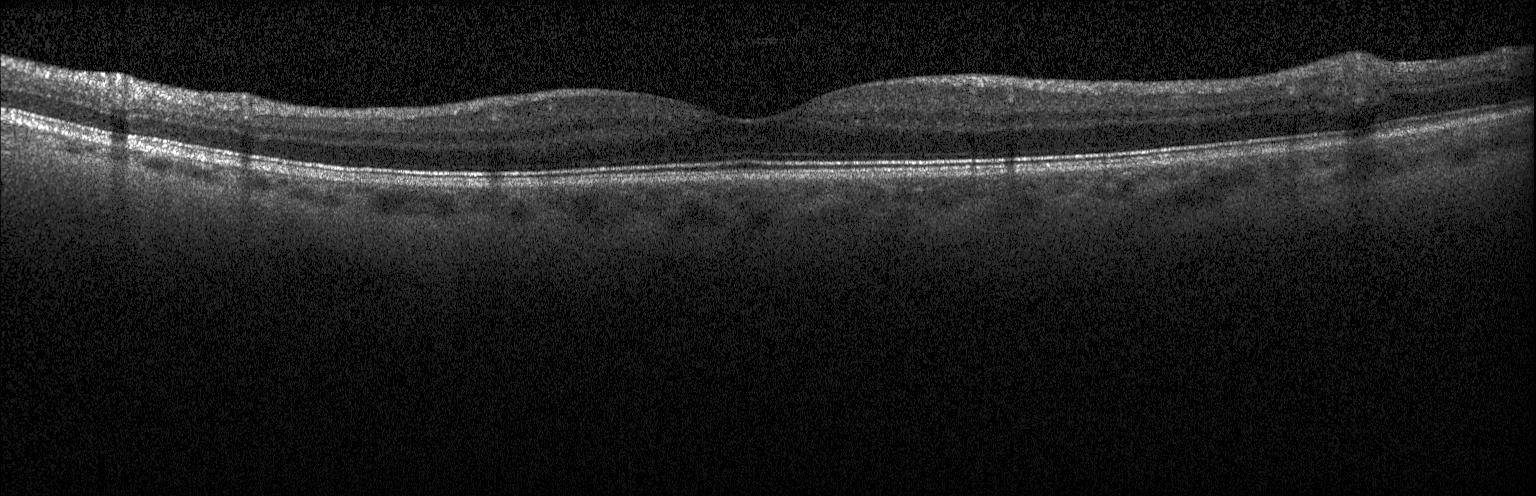

OCT finding: no evidence of choroidal neovascularization, diabetic macular edema, or drusen.